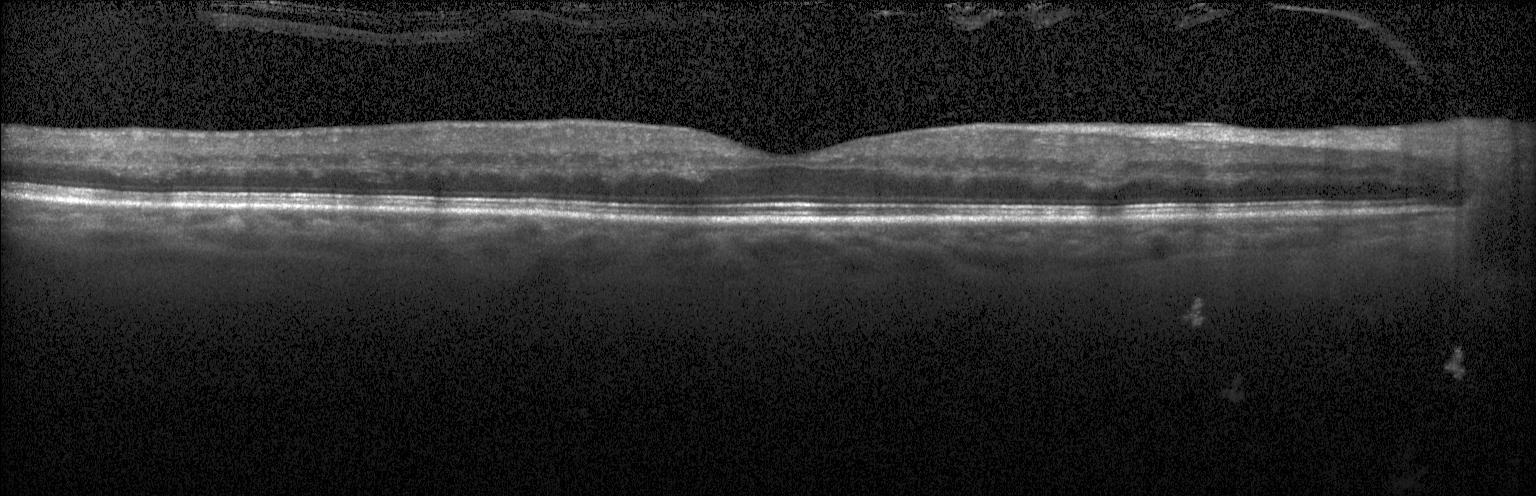 Assessment: neither choroidal neovascularization, diabetic macular edema, nor drusen.